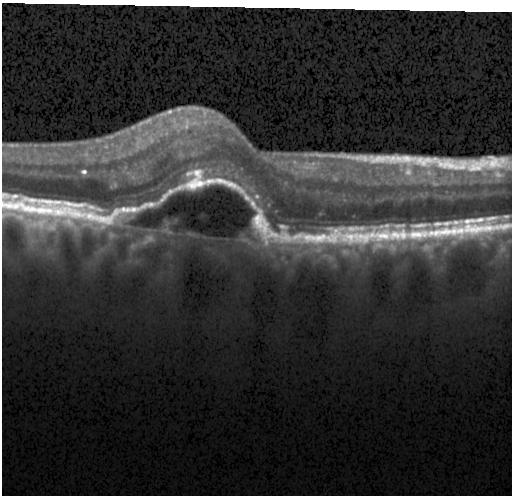
OCT finding: choroidal neovascularization (CNV).